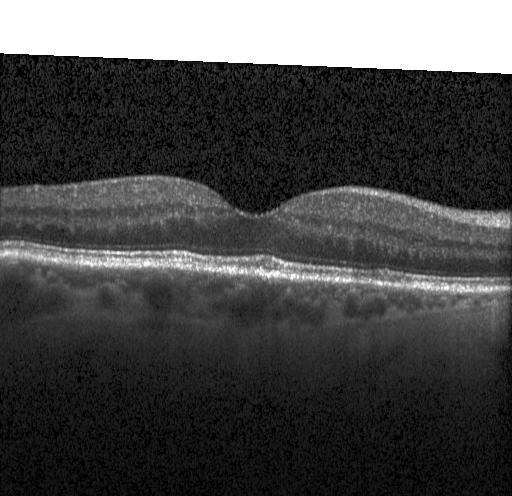
Heidelberg Spectralis. OCT B-scan. Centered on the fovea. SD-OCT
Diagnosis: no choroidal neovascularization, diabetic macular edema, or drusen.